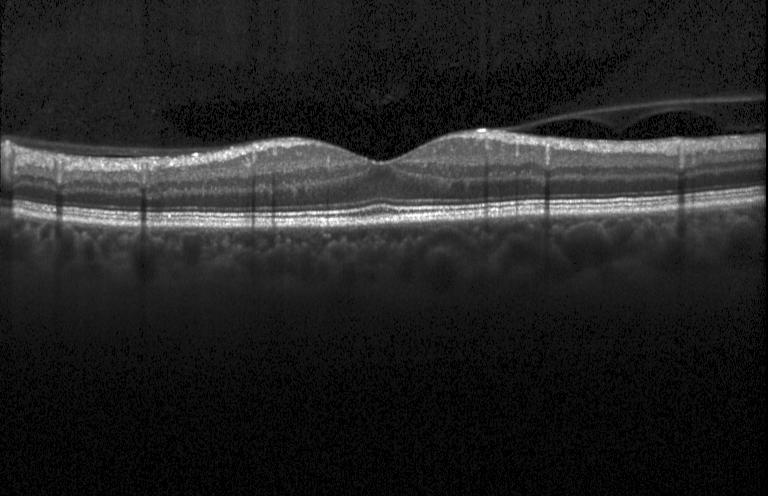

This B-scan demonstrates no choroidal neovascularization, no diabetic macular edema, and no drusen.